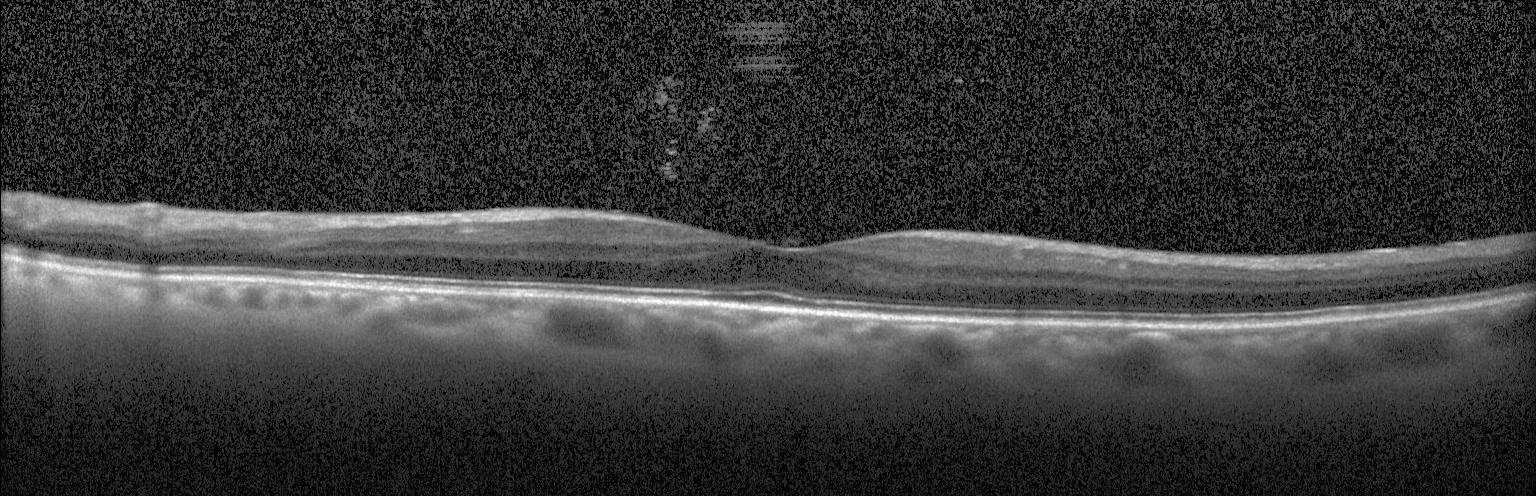
Retinal OCT cross-section, spectral-domain OCT. Macular OCT: no choroidal neovascularization, no diabetic macular edema, and no drusen.